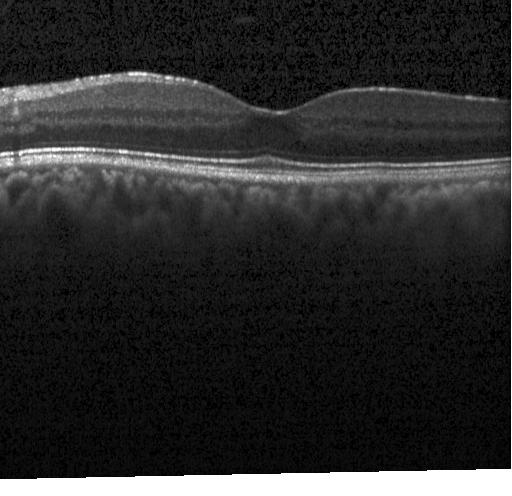

Retinal OCT cross-section — Neither choroidal neovascularization, diabetic macular edema, nor drusen.